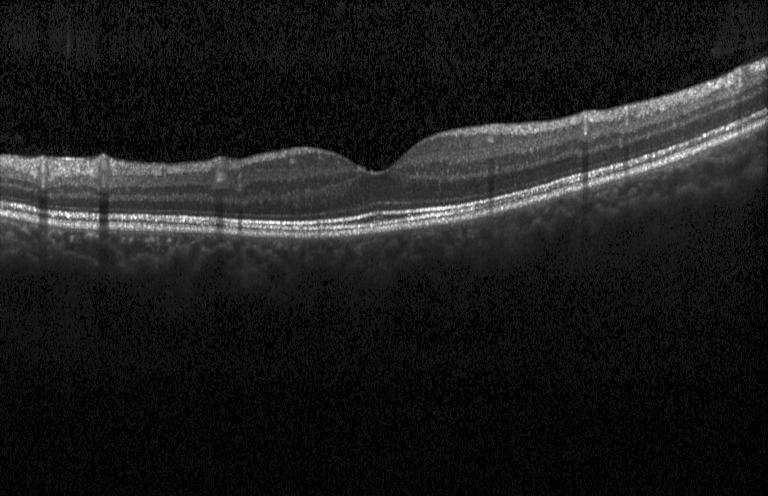

Retinal OCT cross-section.
Dx: no evidence of choroidal neovascularization, diabetic macular edema, or drusen.